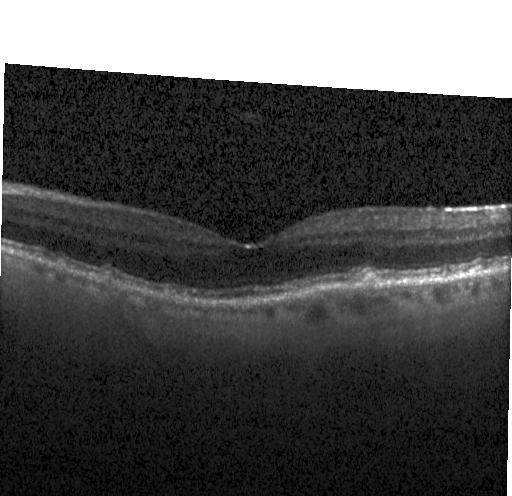 Centered on the fovea · Heidelberg Spectralis OCT system · SD-OCT · optical coherence tomography scan. Finding: drusen.